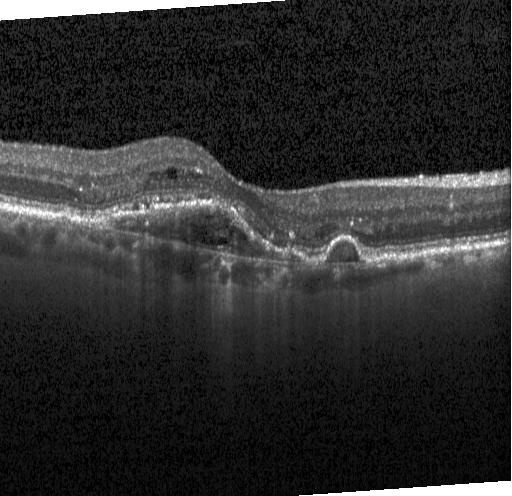

Spectral-domain OCT; OCT B-scan; horizontal scan through the fovea.
OCT finding: a choroidal neovascular membrane.